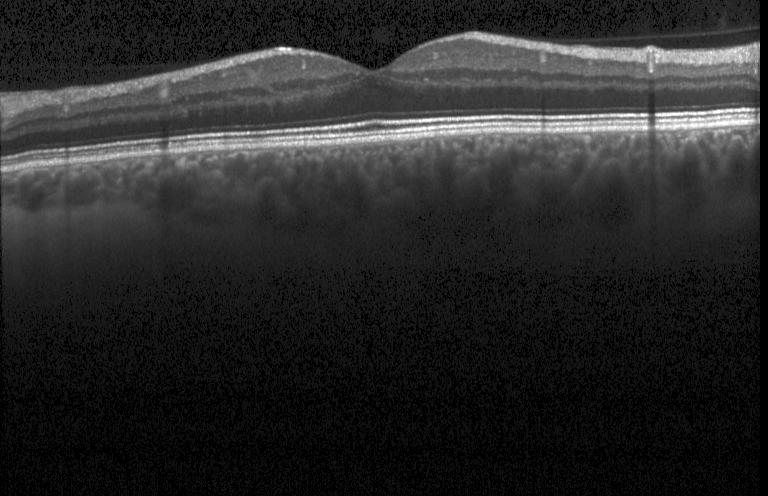

OCT line scan — Finding: no evidence of choroidal neovascularization, diabetic macular edema, or drusen.